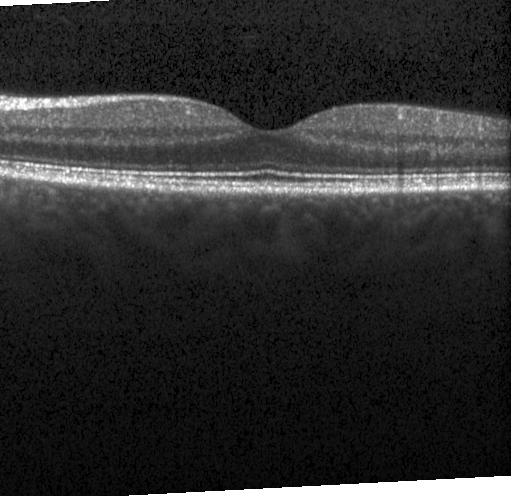
Optical coherence tomography scan — Assessment: no CNV, no DME, and no drusen.